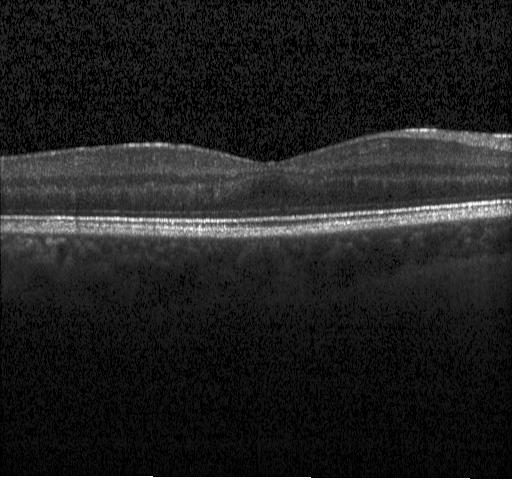
SD-OCT · acquired on a Heidelberg Spectralis · optical coherence tomography scan · macular scan.
Finding: no CNV, DME, or drusen.